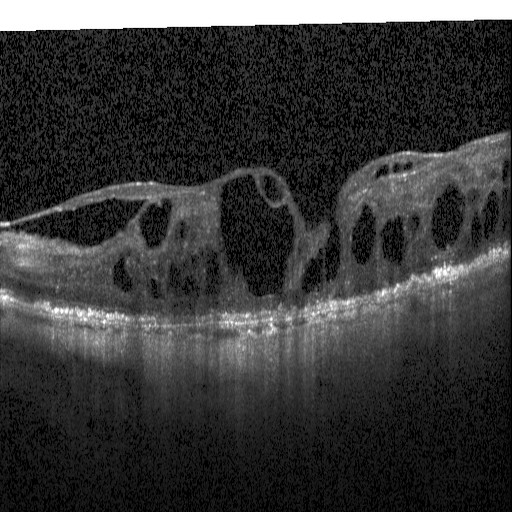
Diagnosis: diabetic macular edema (DME).